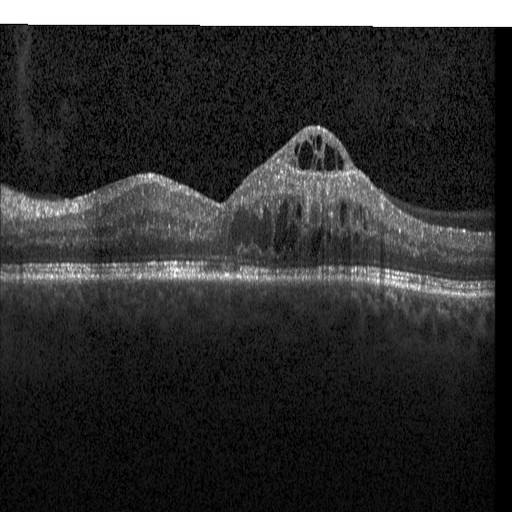 Retinal OCT cross-section · spectral-domain OCT
Finding: DME.